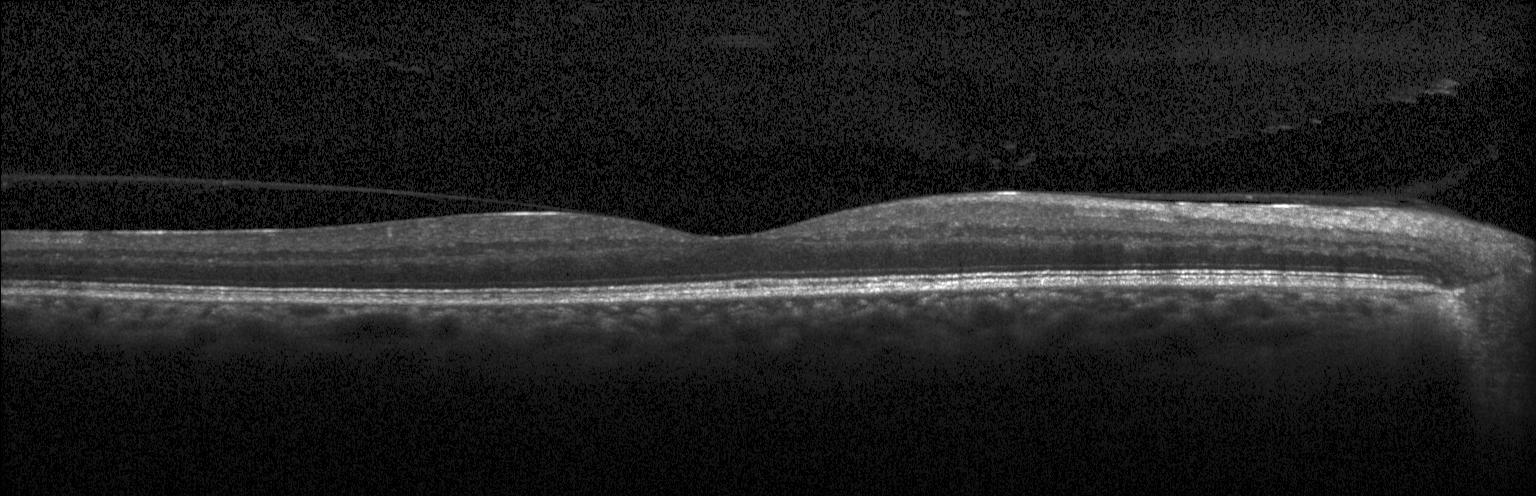 Retinal OCT cross-section. No evidence of choroidal neovascularization, diabetic macular edema, or drusen.